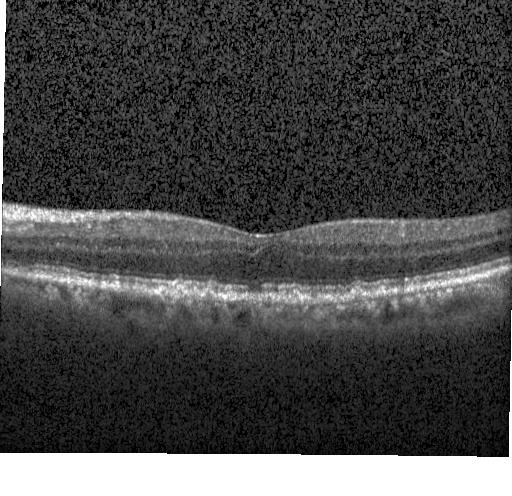 Spectral-domain optical coherence tomography · optical coherence tomography B-scan — Assessment: multiple drusen.